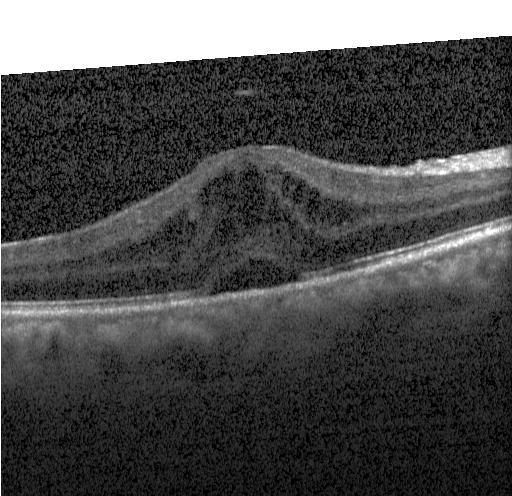 Retinal OCT B-scan.
The scan shows DME.